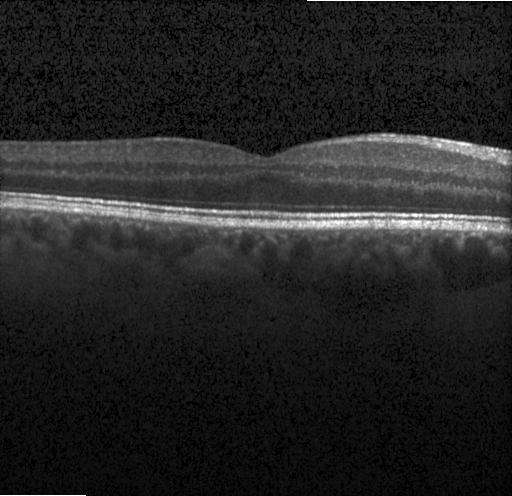
OCT line scan.
Finding: neither choroidal neovascularization, diabetic macular edema, nor drusen.